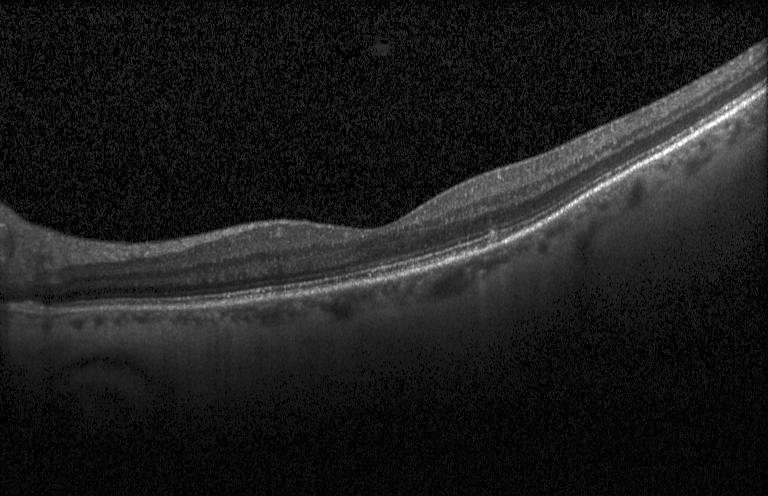 Optical coherence tomography scan, SD-OCT
No evidence of choroidal neovascularization, diabetic macular edema, or drusen.